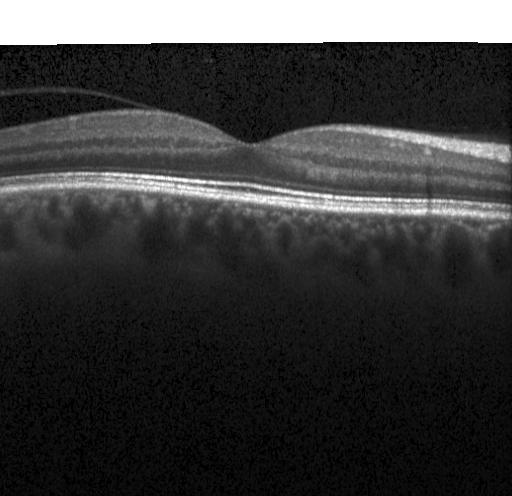
OCT B-scan showing no evidence of choroidal neovascularization, diabetic macular edema, or drusen.